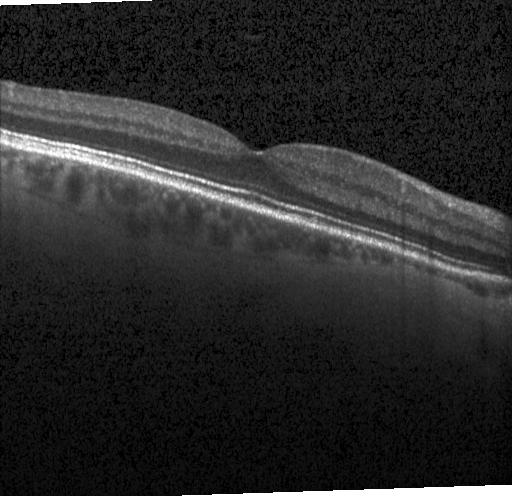 OCT B-scan; horizontal scan through the fovea; instrument: Heidelberg Spectralis. This B-scan demonstrates no evidence of choroidal neovascularization, diabetic macular edema, or drusen.